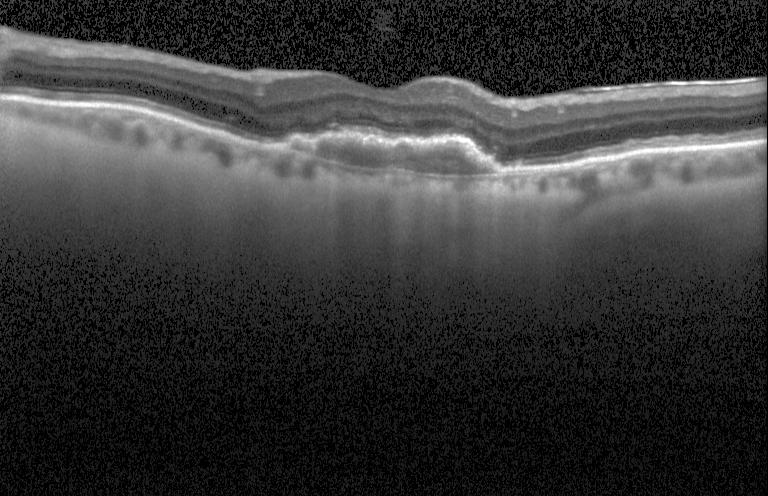

A choroidal neovascular membrane.